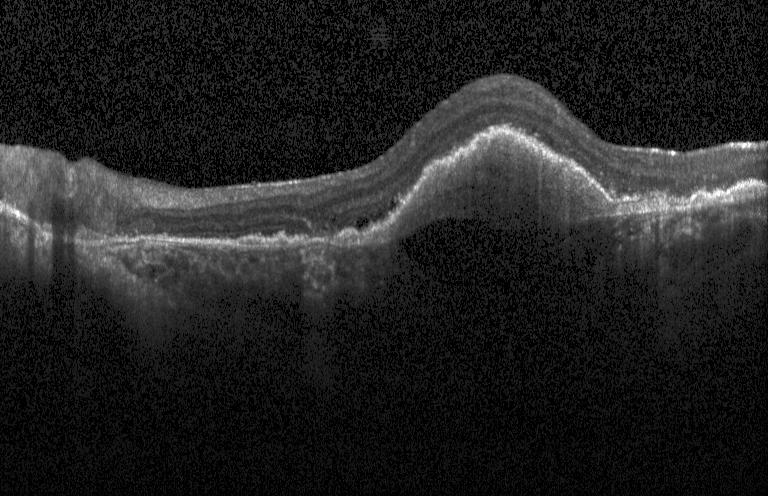
Spectral-domain optical coherence tomography; optical coherence tomography B-scan; Heidelberg Spectralis; macular scan.
CNV.